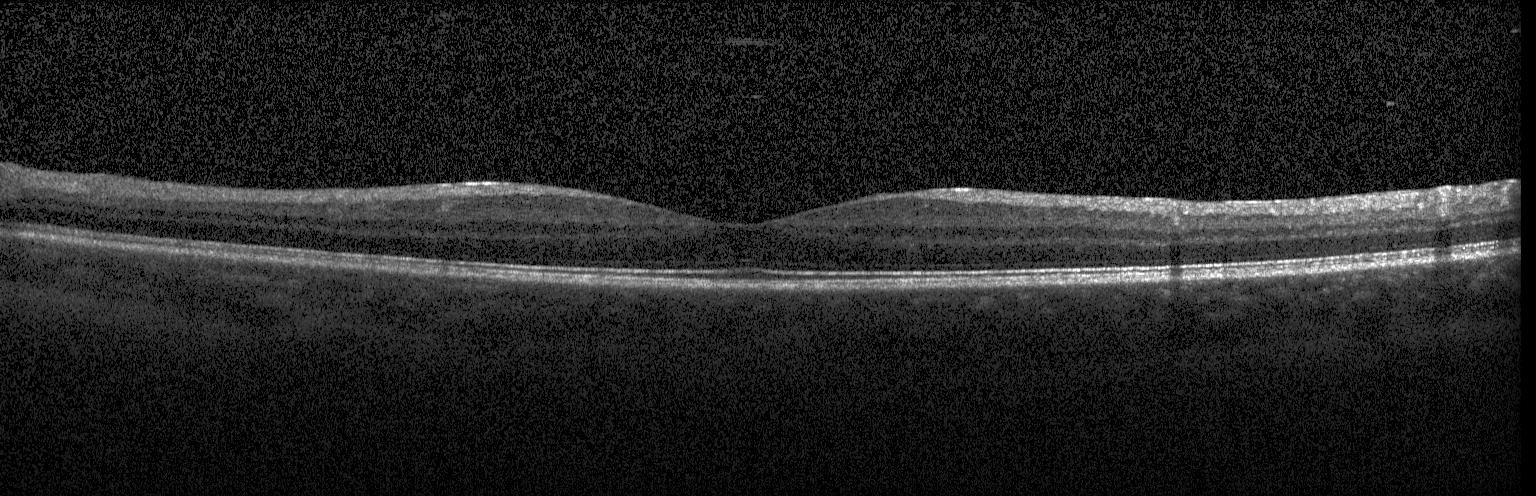 OCT finding: neither choroidal neovascularization, diabetic macular edema, nor drusen.